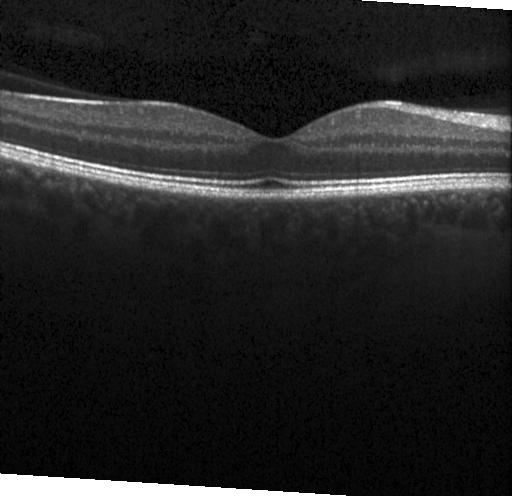
Horizontal scan through the fovea. Optical coherence tomography B-scan. Acquired on a Heidelberg Spectralis. Finding: neither CNV, DME, nor drusen.